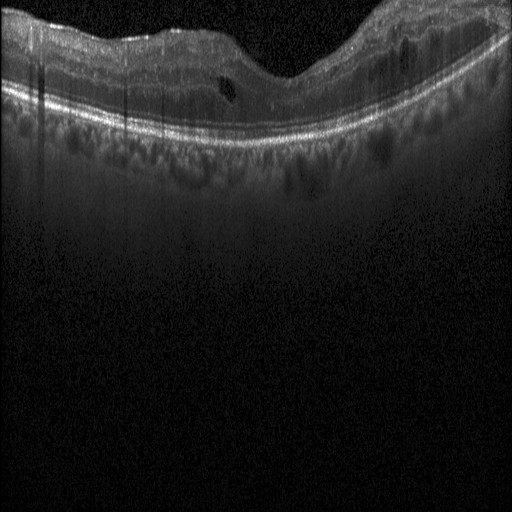 Impression: diabetic macular edema (DME).